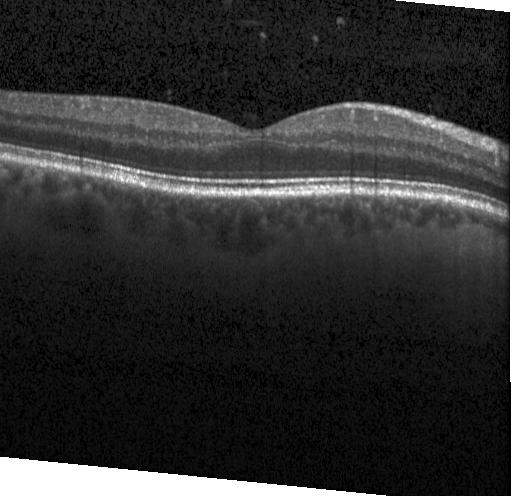 Macular scan; Heidelberg Spectralis OCT system; optical coherence tomography scan. This B-scan demonstrates no evidence of choroidal neovascularization, diabetic macular edema, or drusen.